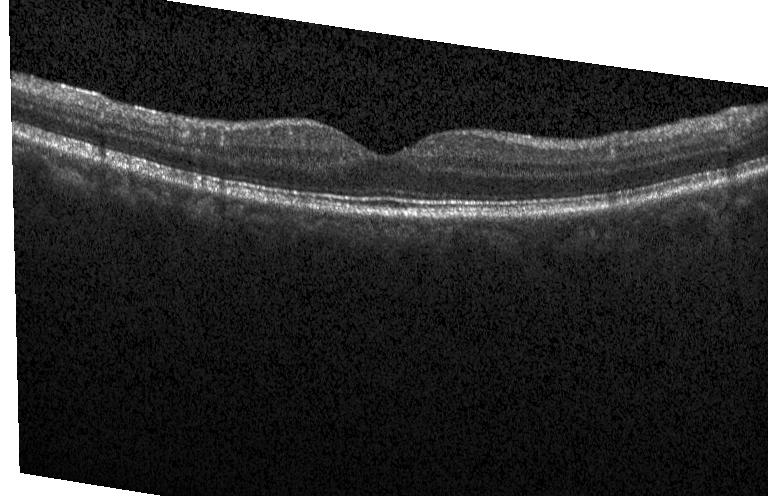 OCT scan showing no choroidal neovascularization, no diabetic macular edema, and no drusen.